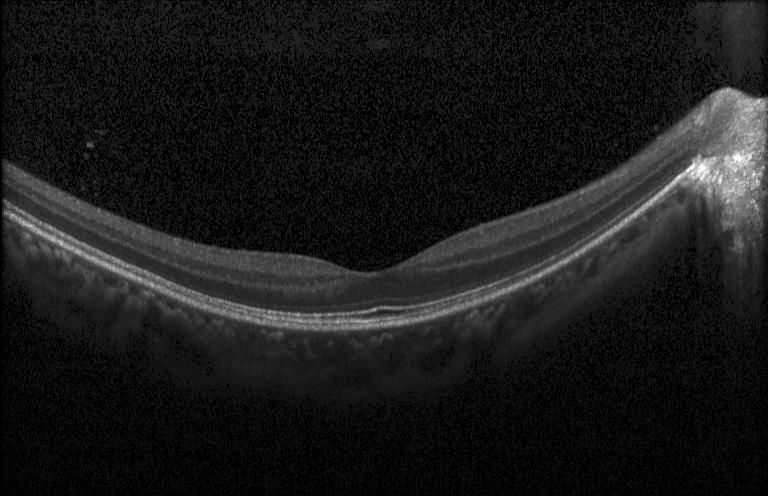 This B-scan demonstrates no choroidal neovascularization, no diabetic macular edema, and no drusen.